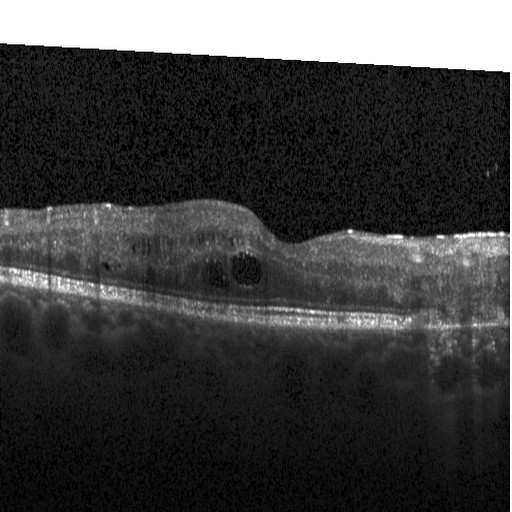
Dx: diabetic macular edema.